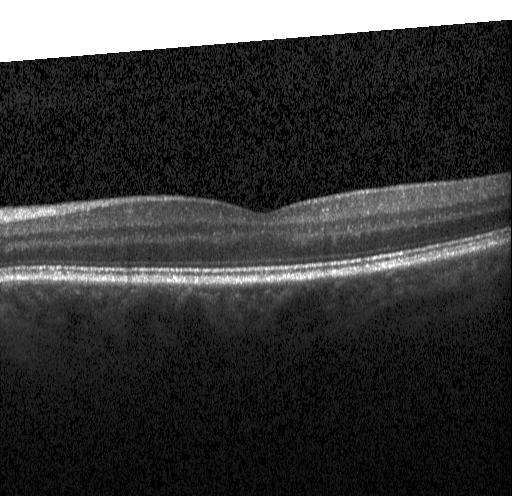
Diagnosis: no evidence of choroidal neovascularization, diabetic macular edema, or drusen.